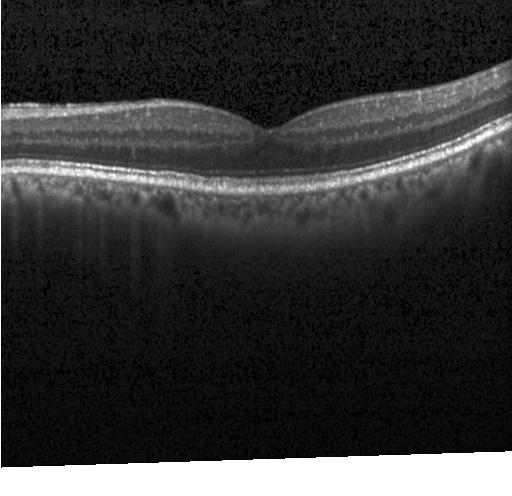 Optical coherence tomography scan; spectral-domain optical coherence tomography
Diagnosis: no choroidal neovascularization, diabetic macular edema, or drusen.